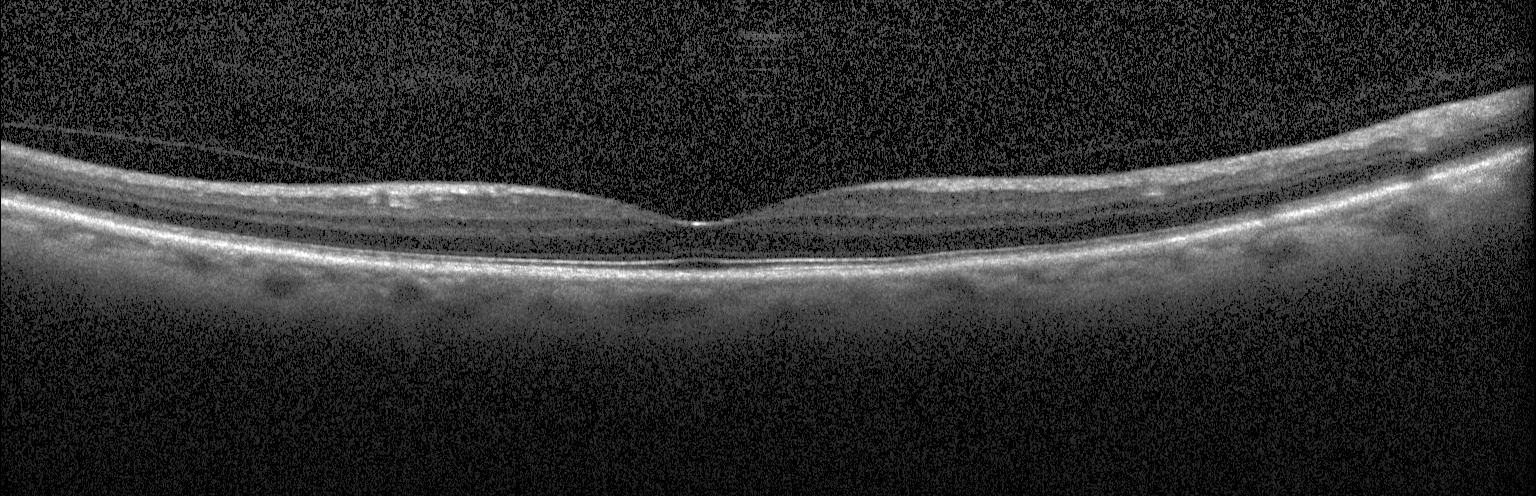 Instrument: Heidelberg Spectralis · optical coherence tomography scan · centered on the fovea · spectral-domain OCT.
This B-scan demonstrates no choroidal neovascularization, no diabetic macular edema, and no drusen.